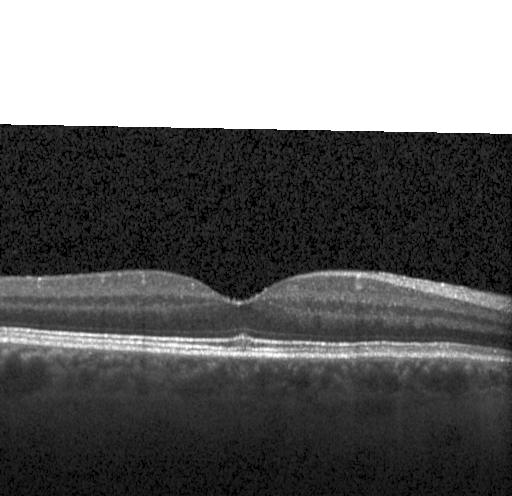

No evidence of choroidal neovascularization, diabetic macular edema, or drusen.